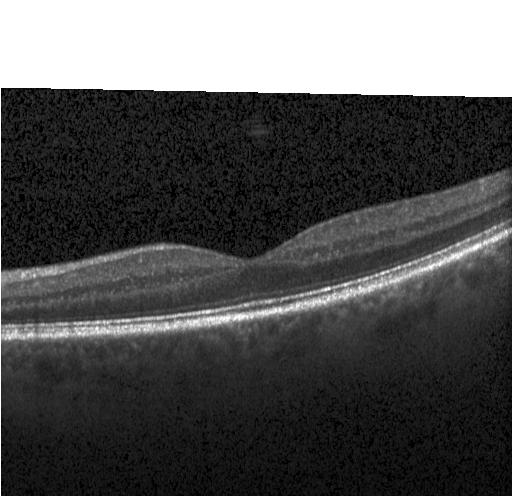 Instrument: Heidelberg Spectralis; OCT B-scan
Diagnosis: no choroidal neovascularization, no diabetic macular edema, and no drusen.